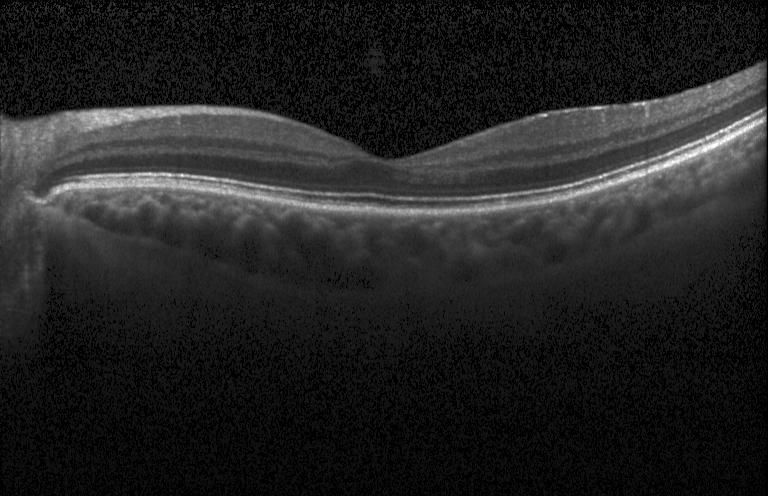
Fovea-centered, OCT B-scan. The scan shows no CNV, DME, or drusen.